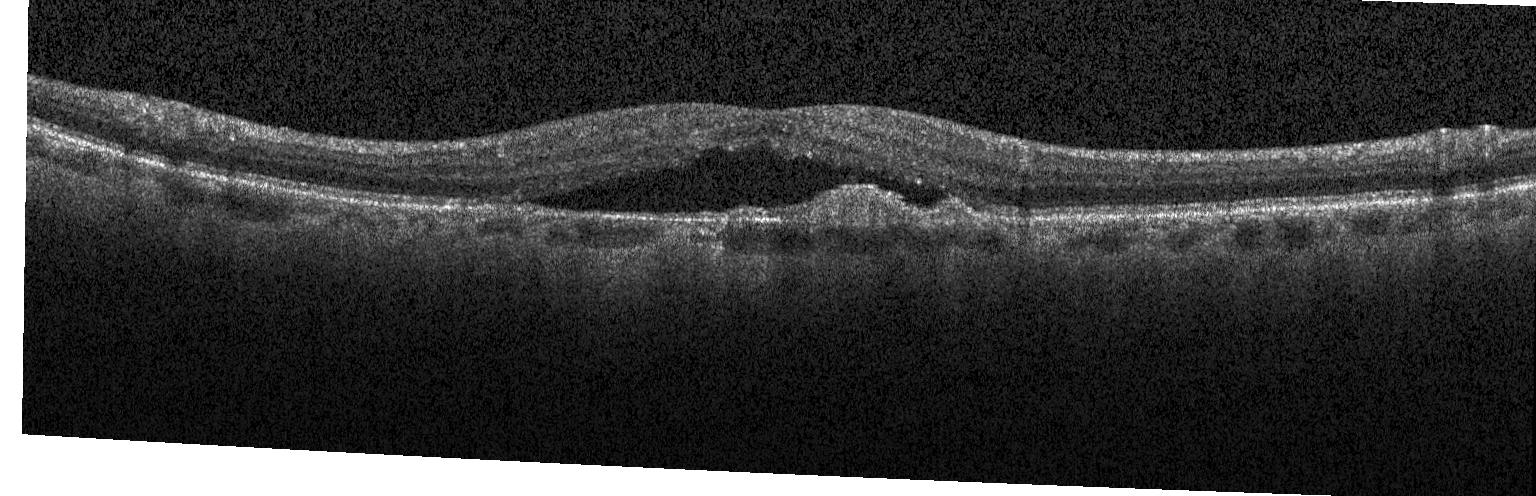 CNV.